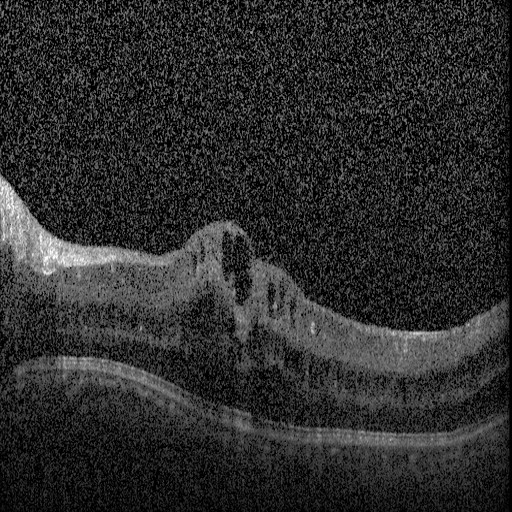 Finding: diabetic macular edema.